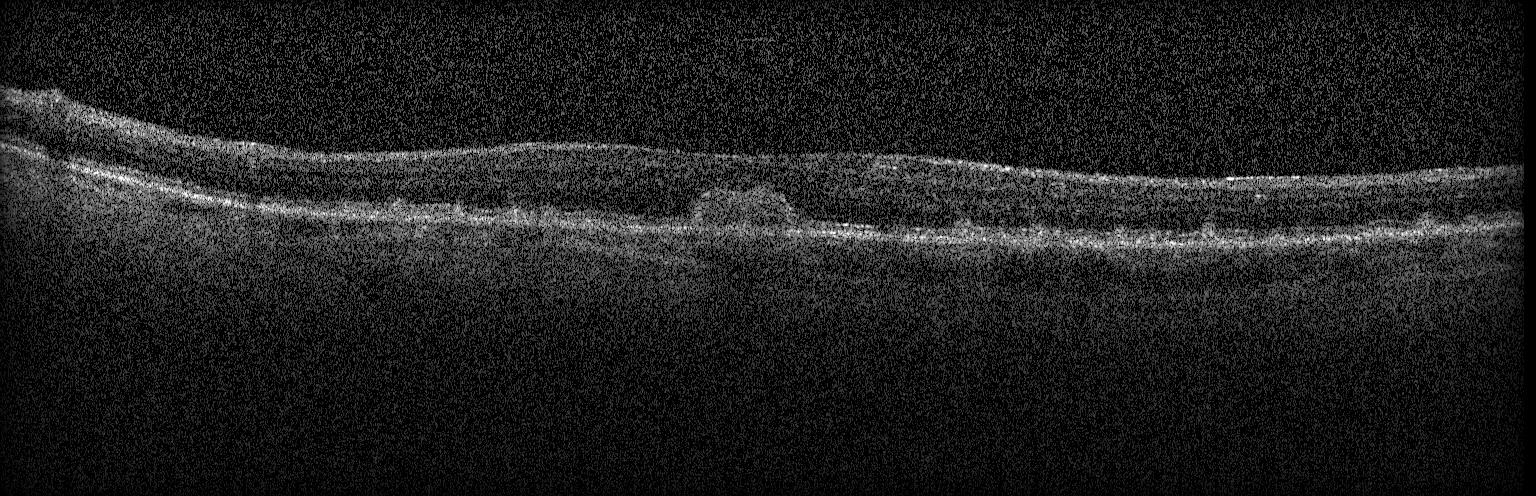
The scan shows a choroidal neovascular membrane.